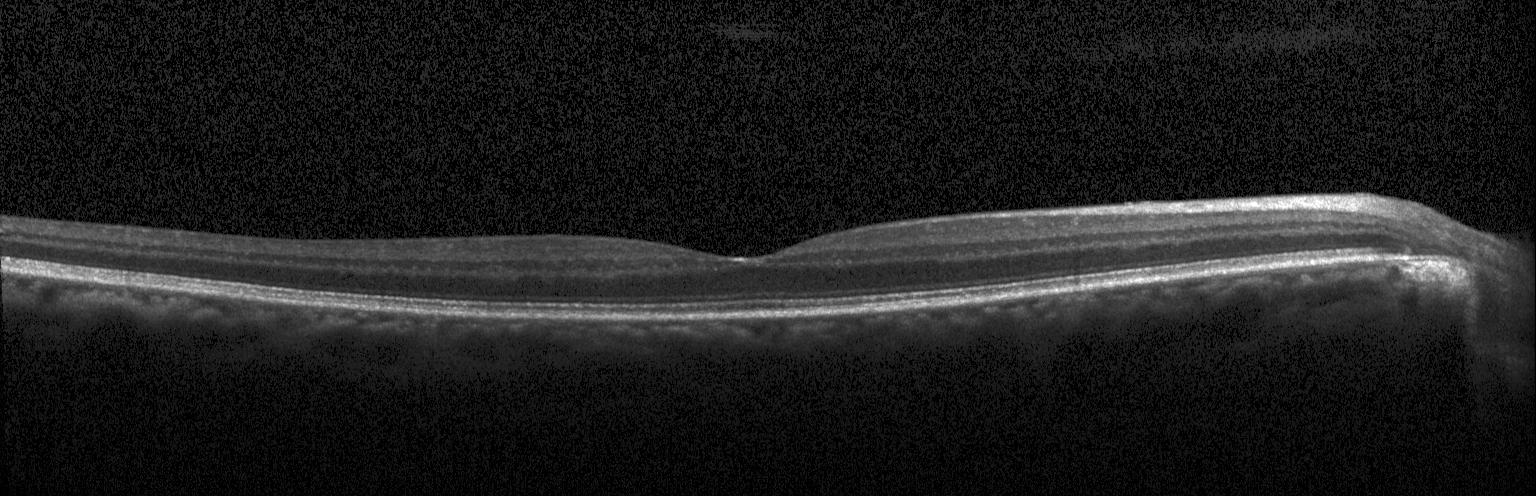 This B-scan demonstrates no choroidal neovascularization, diabetic macular edema, or drusen.